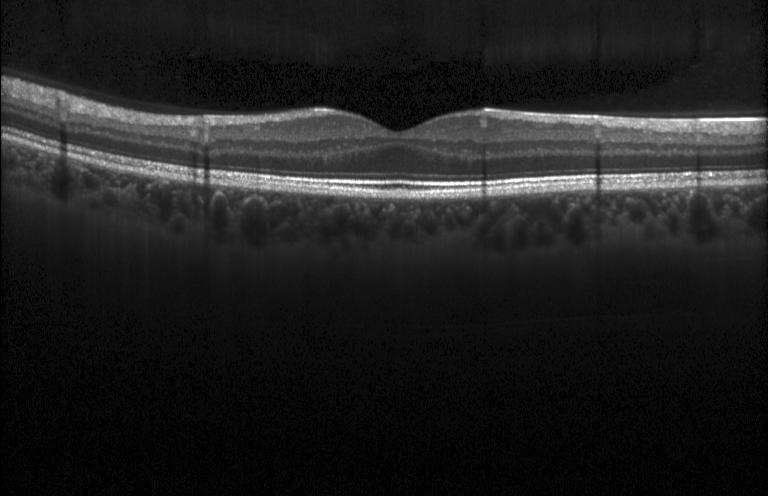 Assessment: no choroidal neovascularization, no diabetic macular edema, and no drusen.